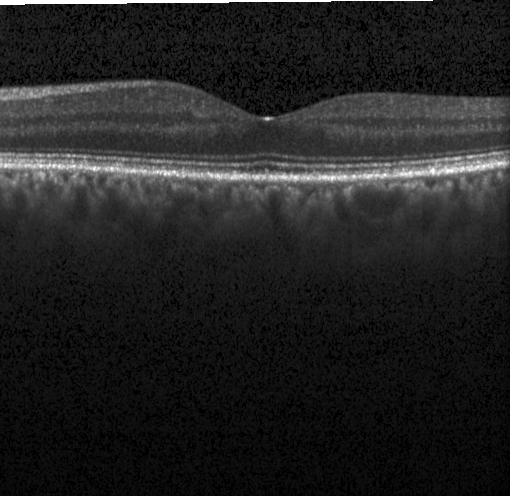 Finding: no choroidal neovascularization, diabetic macular edema, or drusen.